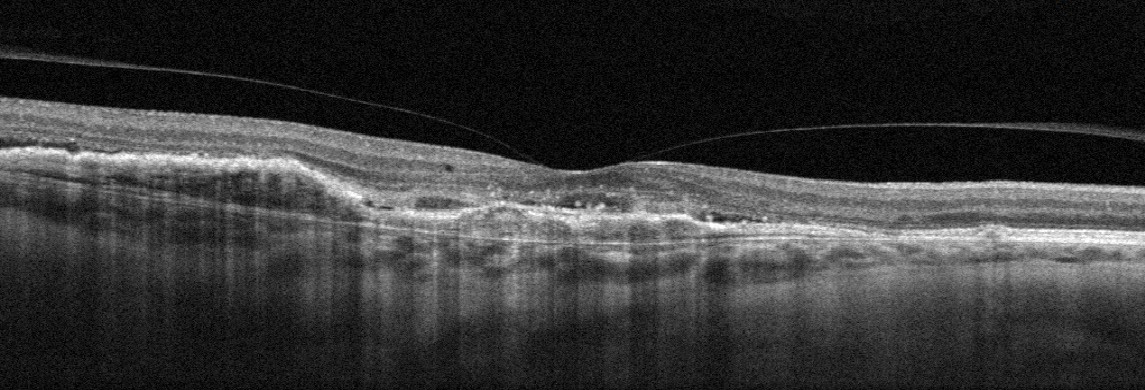 Impression: AMD.